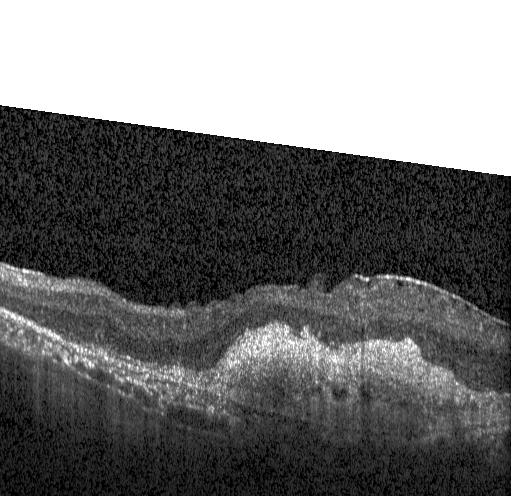
Macular OCT demonstrating choroidal neovascularization.